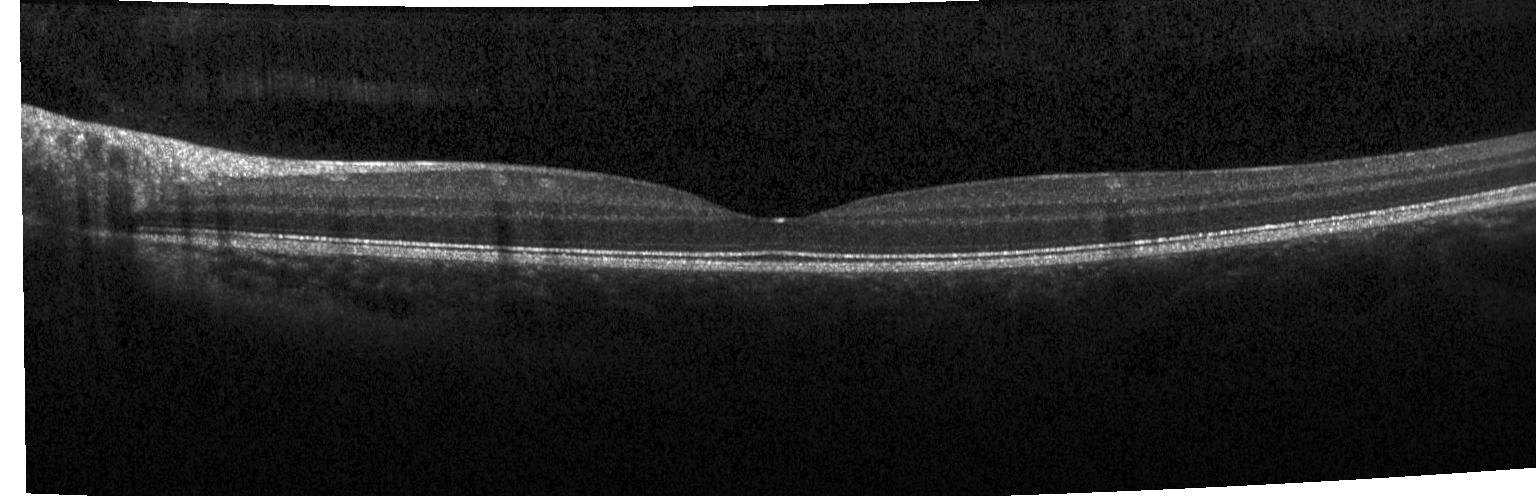 Assessment: neither choroidal neovascularization, diabetic macular edema, nor drusen.